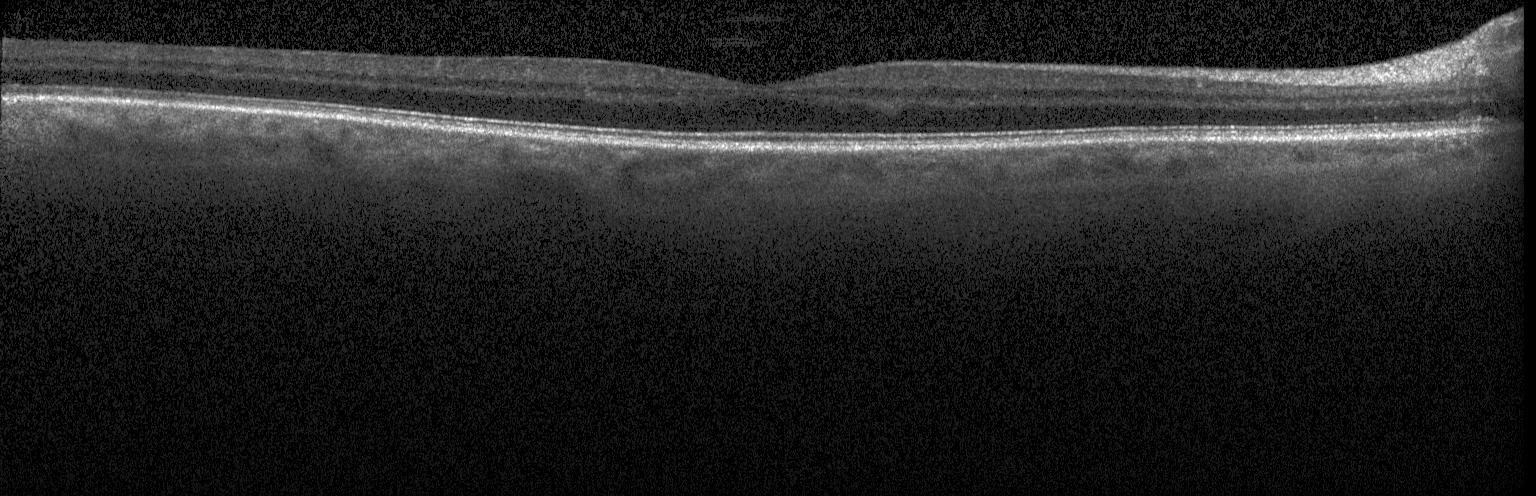 Assessment: no choroidal neovascularization, diabetic macular edema, or drusen.